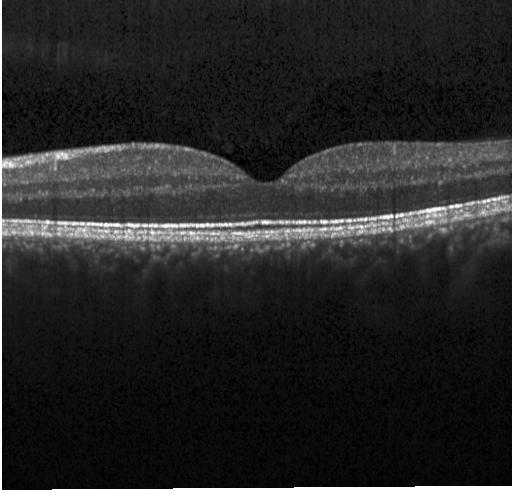 OCT line scan.
Dx: no evidence of choroidal neovascularization, diabetic macular edema, or drusen.